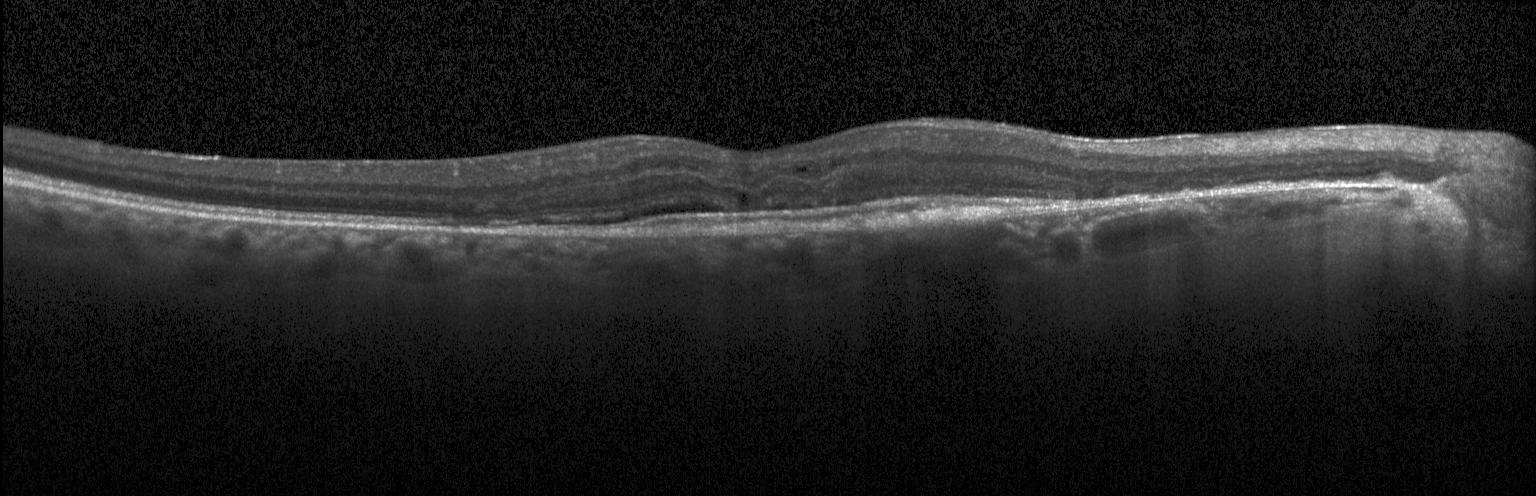 Optical coherence tomography B-scan — Assessment: a choroidal neovascular membrane.